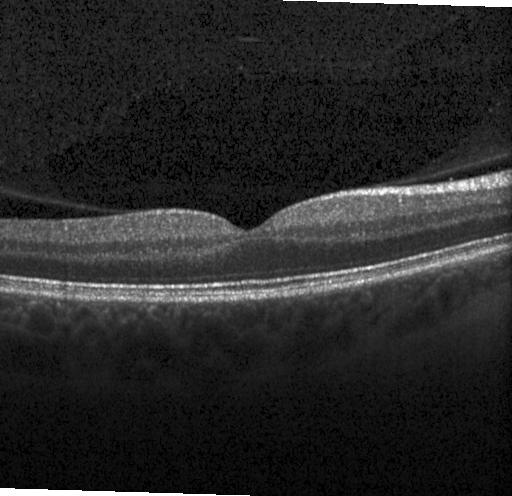
Retinal OCT cross-section
The scan shows no CNV, no DME, and no drusen.